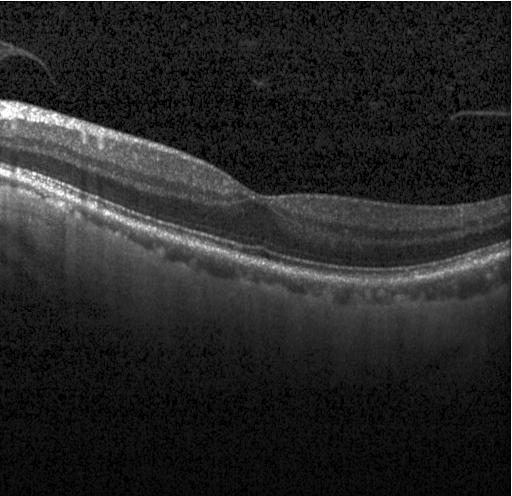 Heidelberg Spectralis OCT system; horizontal scan through the fovea; retinal OCT cross-section; spectral-domain optical coherence tomography.
Dx: no evidence of choroidal neovascularization, diabetic macular edema, or drusen.